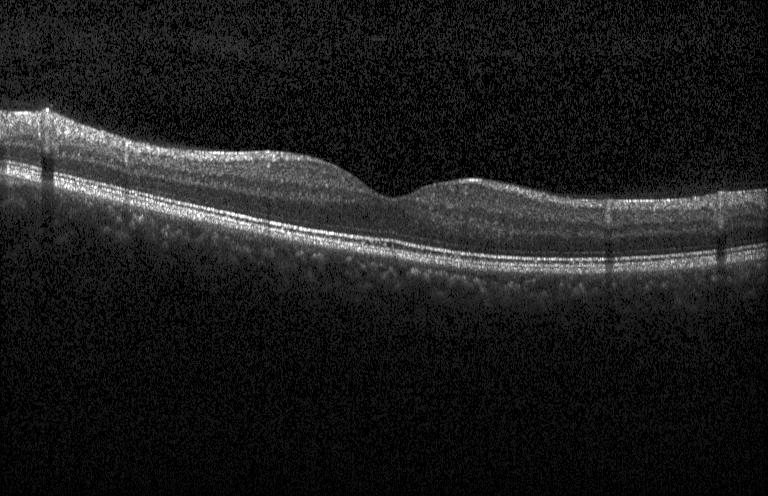
Impression: neither CNV, DME, nor drusen.